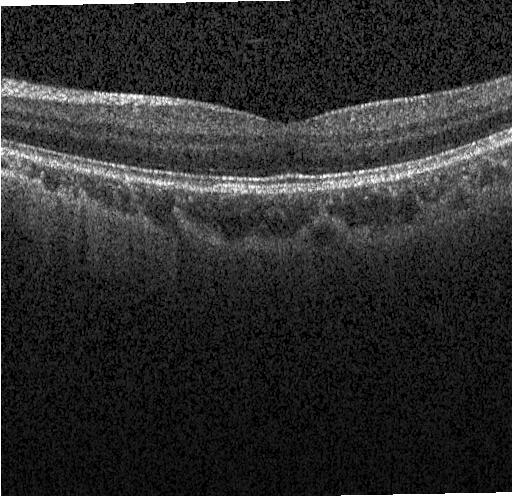 Macular OCT demonstrating no evidence of CNV, DME, or drusen.